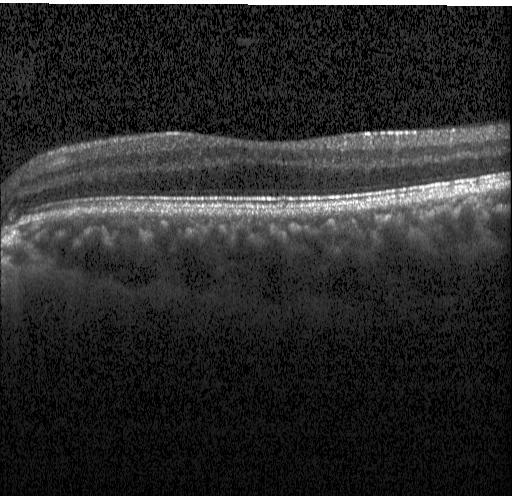 SD-OCT · OCT line scan · centered on the fovea
Finding: no evidence of choroidal neovascularization, diabetic macular edema, or drusen.